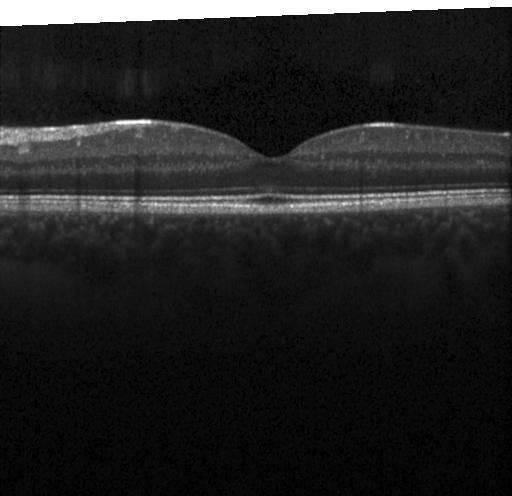 Optical coherence tomography scan
Impression: no evidence of choroidal neovascularization, diabetic macular edema, or drusen.